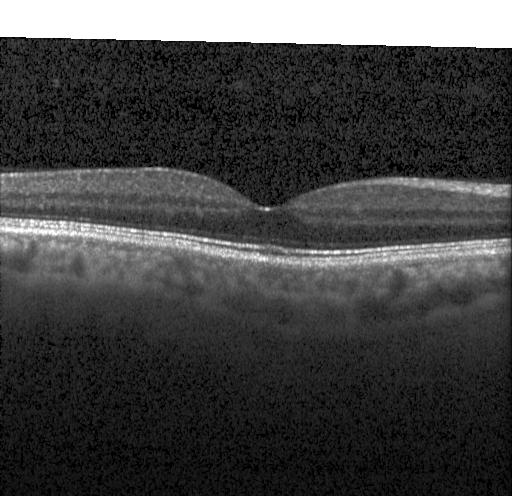
OCT line scan. The scan shows no evidence of CNV, DME, or drusen.